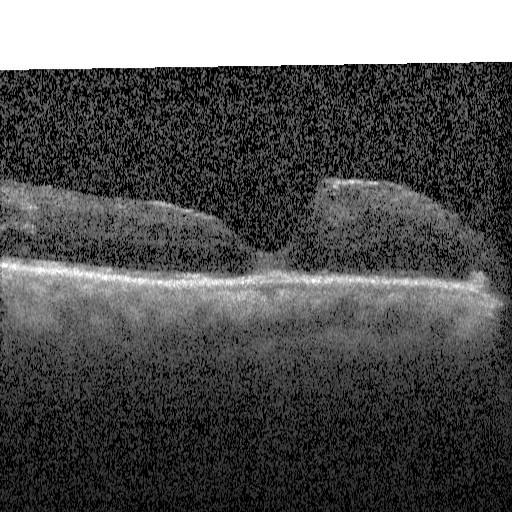 Optical coherence tomography scan. SD-OCT.
Impression: DME.